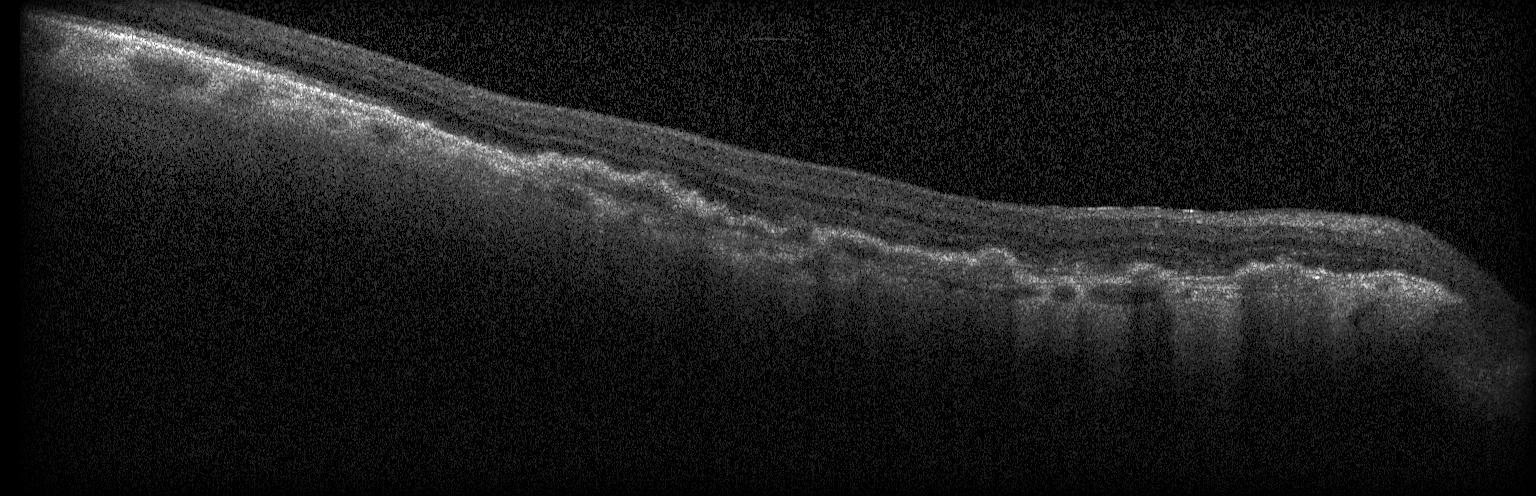

OCT B-scan.
Diagnosis: choroidal neovascularization (CNV).